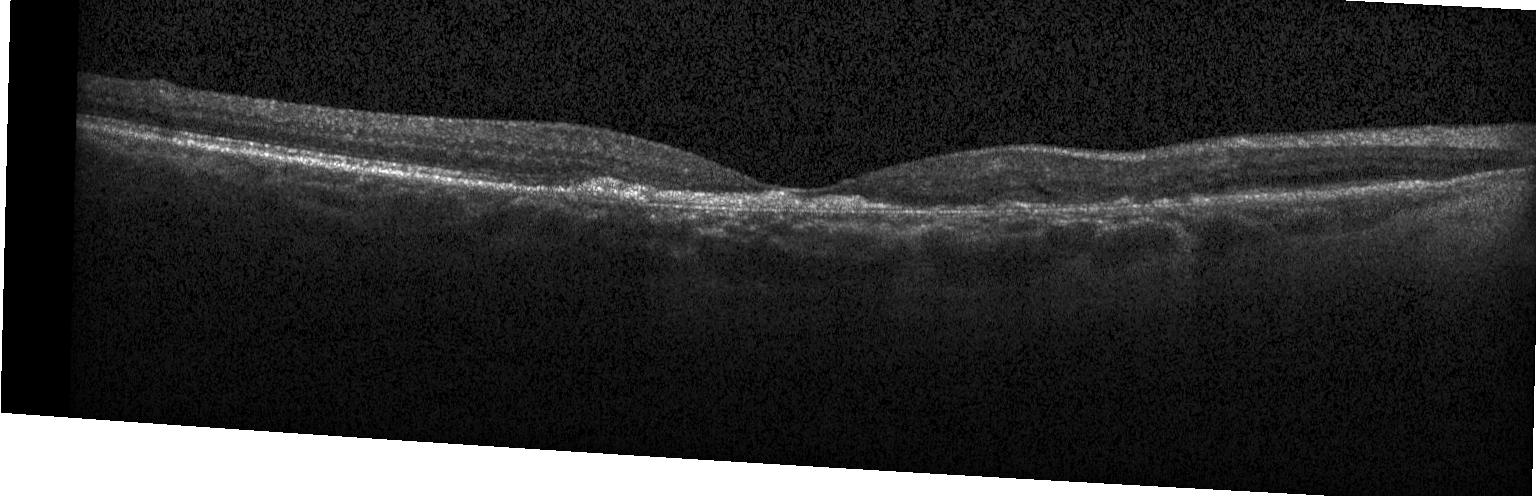
Macular OCT: choroidal neovascularization (CNV).